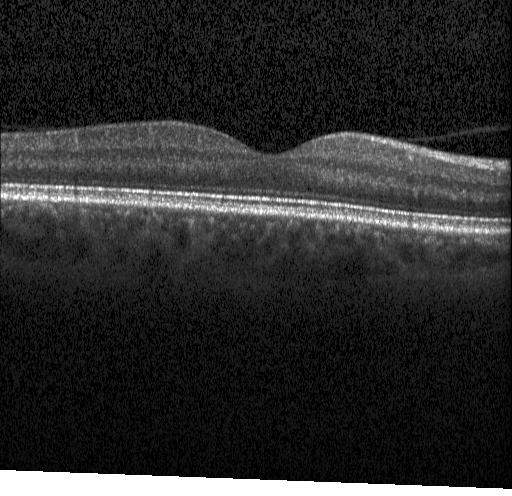 Heidelberg Spectralis OCT system; retinal OCT B-scan; SD-OCT; macular scan
Diagnosis: no evidence of choroidal neovascularization, diabetic macular edema, or drusen.